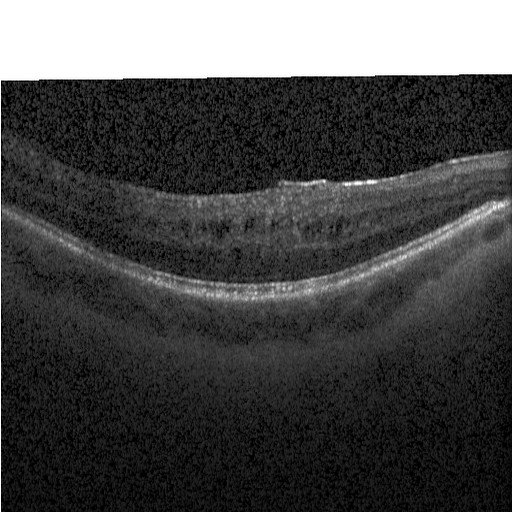 OCT B-scan — Impression: diabetic macular edema (DME).